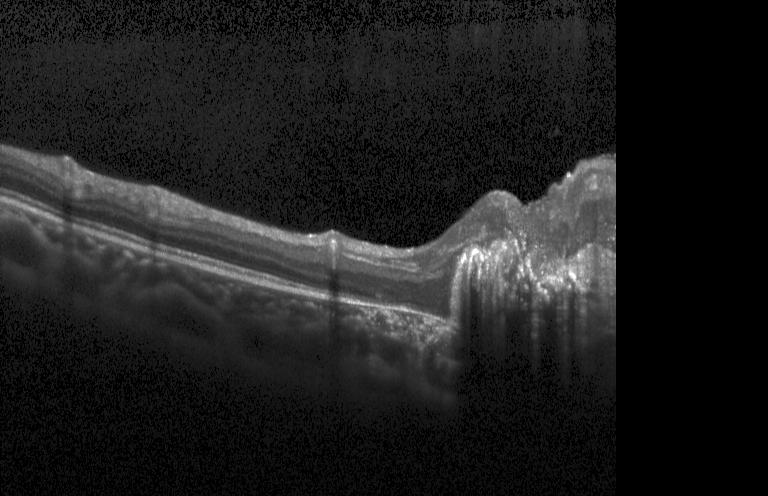
Retinal OCT B-scan — The scan shows a choroidal neovascular membrane.